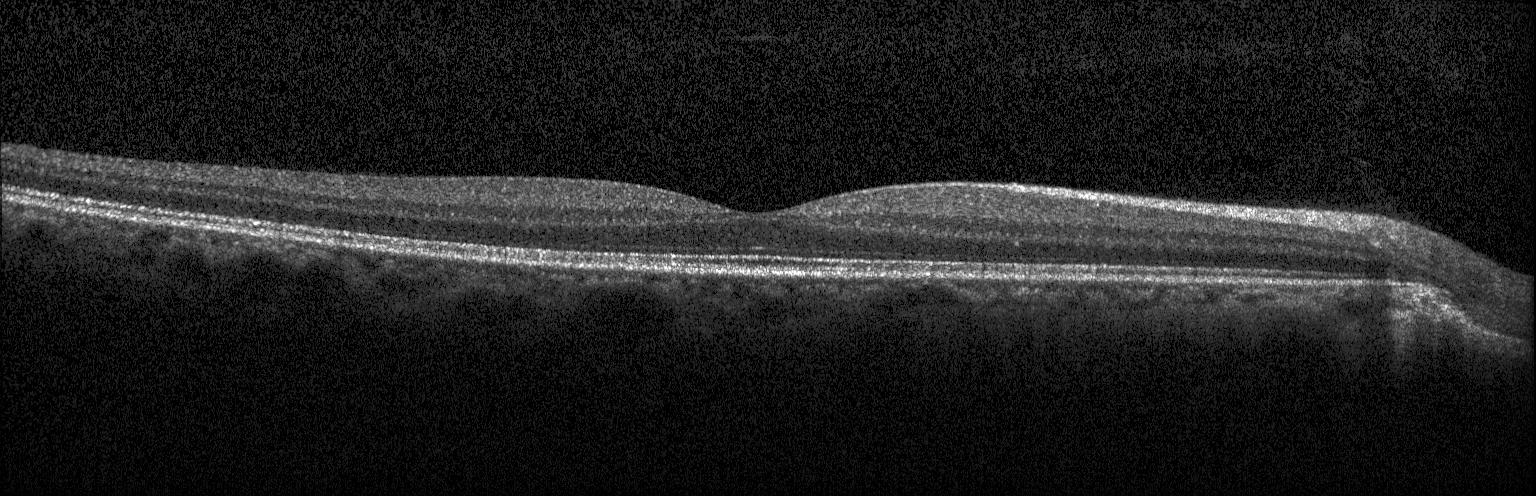 Macular OCT demonstrating neither choroidal neovascularization, diabetic macular edema, nor drusen.